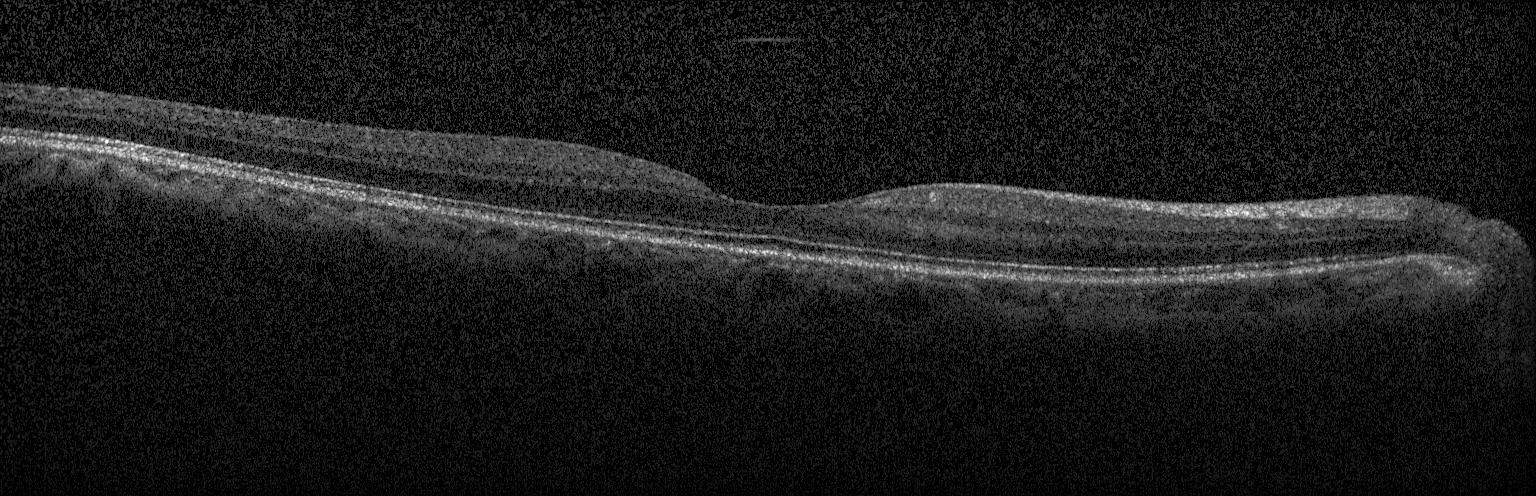

Spectral-domain optical coherence tomography; retinal OCT cross-section; Heidelberg Spectralis OCT system
Impression: no choroidal neovascularization, diabetic macular edema, or drusen.